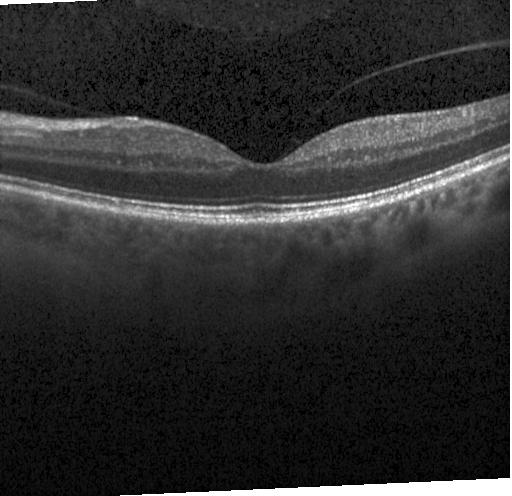

Macular OCT demonstrating no CNV, DME, or drusen.